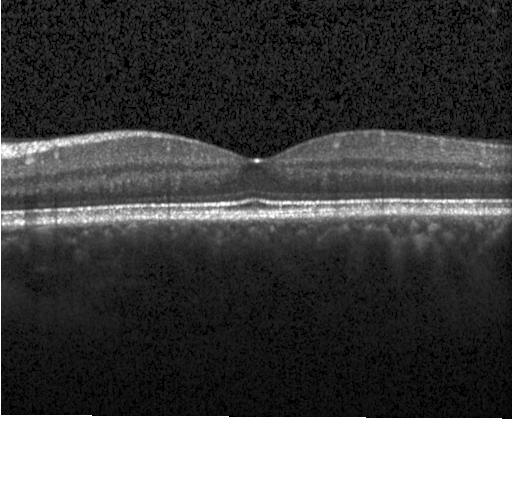 Finding: no evidence of choroidal neovascularization, diabetic macular edema, or drusen.